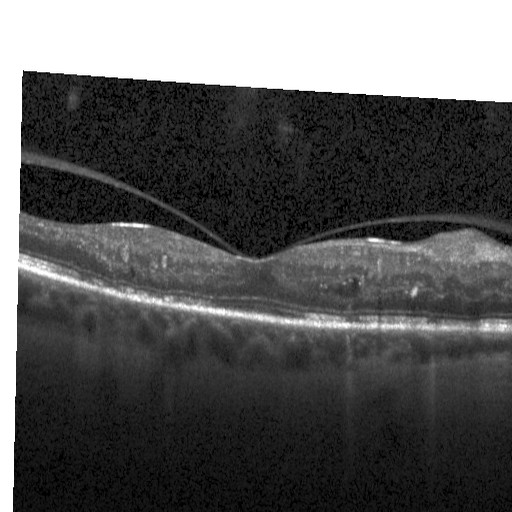
Retinal OCT cross-section — Finding: diabetic macular edema (DME).